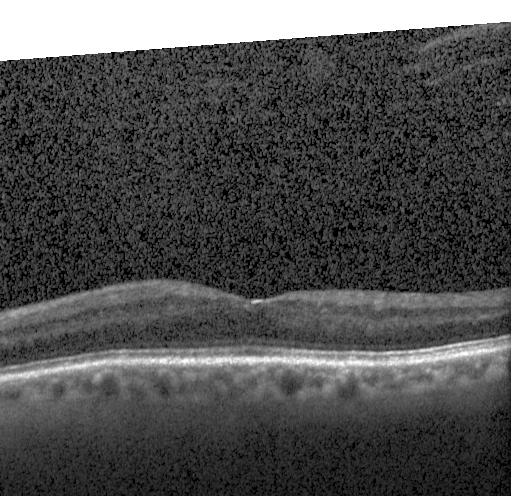

Fovea-centered, SD-OCT, optical coherence tomography B-scan, Heidelberg Spectralis — Assessment: neither choroidal neovascularization, diabetic macular edema, nor drusen.